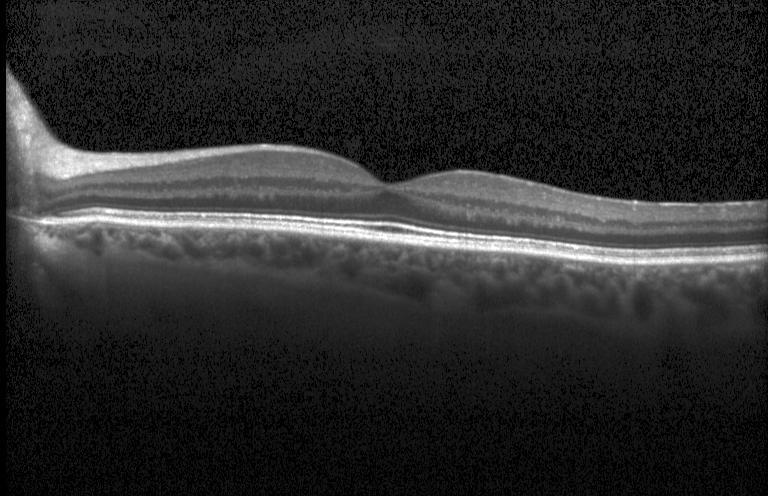

OCT B-scan. Diagnosis: no choroidal neovascularization, no diabetic macular edema, and no drusen.